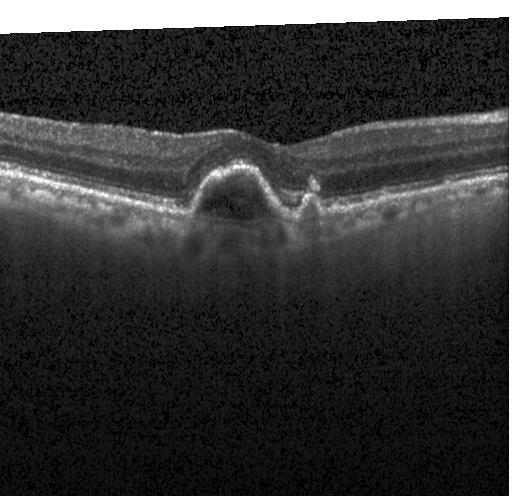
Spectral-domain OCT, retinal OCT cross-section, horizontal scan through the fovea — Impression: a choroidal neovascular membrane.